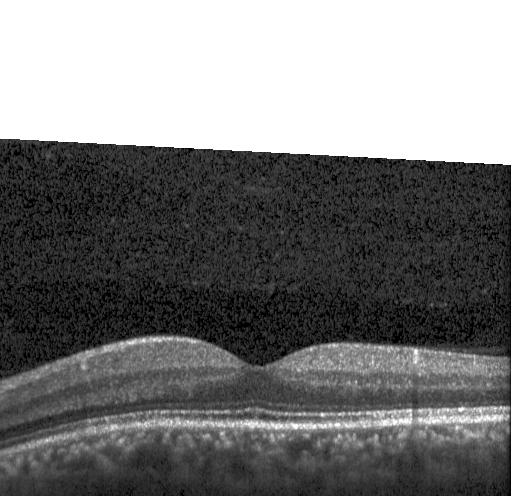
OCT B-scan — Diagnosis: no CNV, no DME, and no drusen.